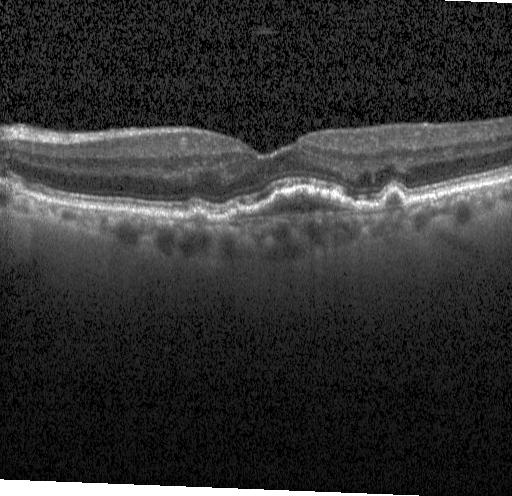 Optical coherence tomography scan · through the macula — This B-scan demonstrates a choroidal neovascular membrane.